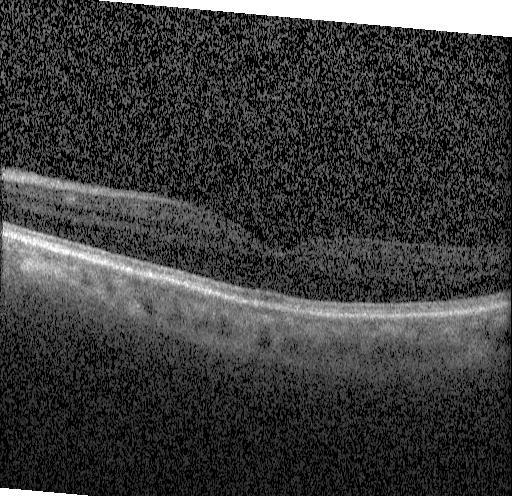
Fovea-centered. Instrument: Heidelberg Spectralis. Spectral-domain OCT. Retinal OCT B-scan — Finding: no CNV, DME, or drusen.